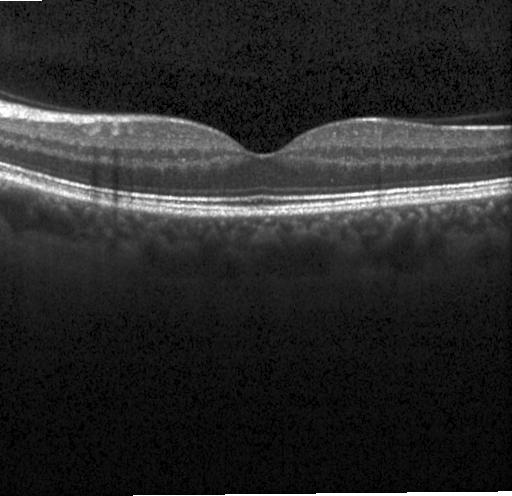

OCT line scan — Diagnosis: no CNV, no DME, and no drusen.